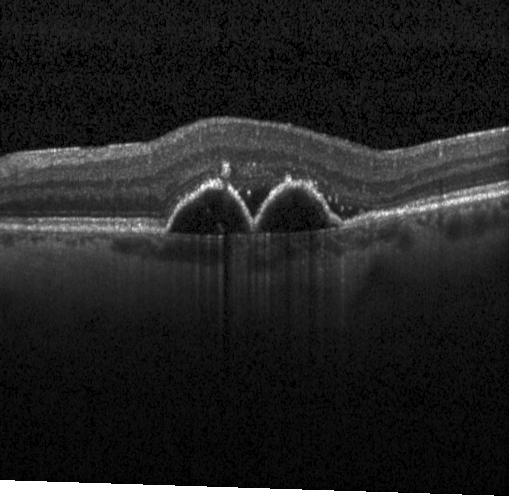

Retinal OCT cross-section, spectral-domain OCT, instrument: Heidelberg Spectralis. Impression: choroidal neovascularization (CNV).